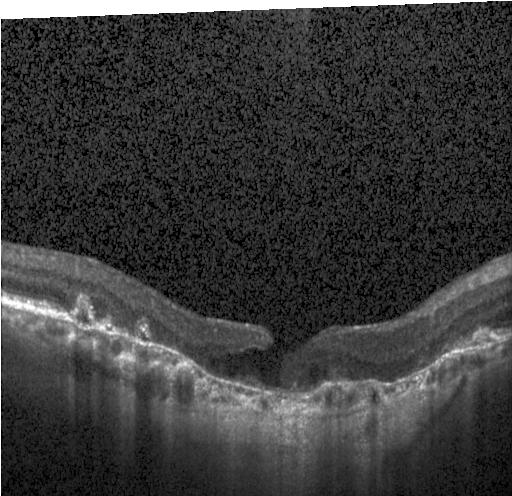 Acquired on a Heidelberg Spectralis, horizontal scan through the fovea, SD-OCT, retinal OCT cross-section
Dx: a choroidal neovascular membrane.